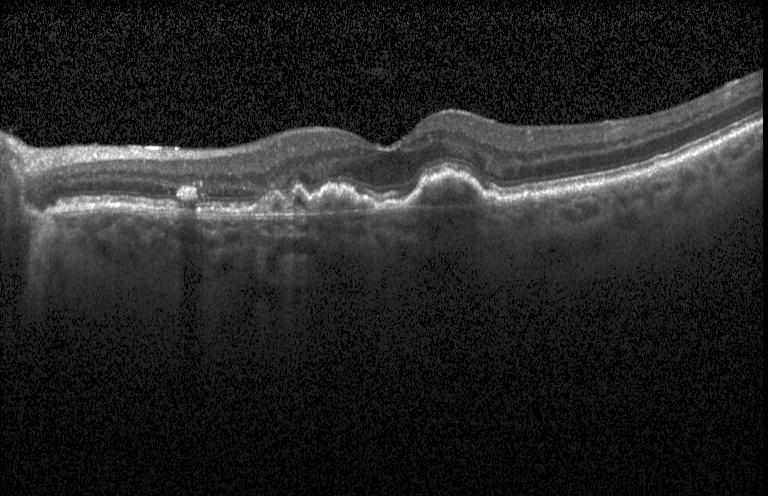

Macular scan · spectral-domain OCT · optical coherence tomography B-scan · acquired on a Heidelberg Spectralis — Dx: a choroidal neovascular membrane.